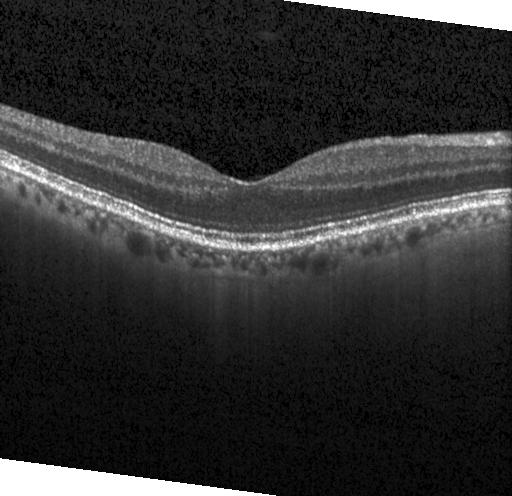
SD-OCT, retinal OCT B-scan, centered on the fovea
Finding: neither CNV, DME, nor drusen.